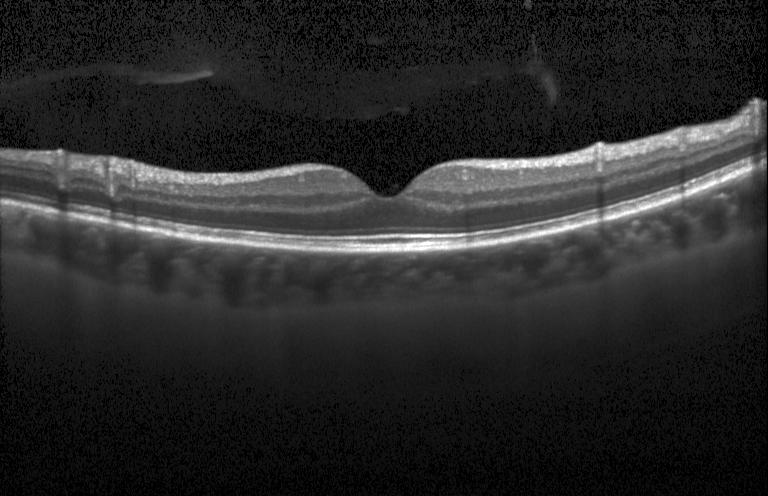

Spectral-domain OCT B-scan: no choroidal neovascularization, no diabetic macular edema, and no drusen.